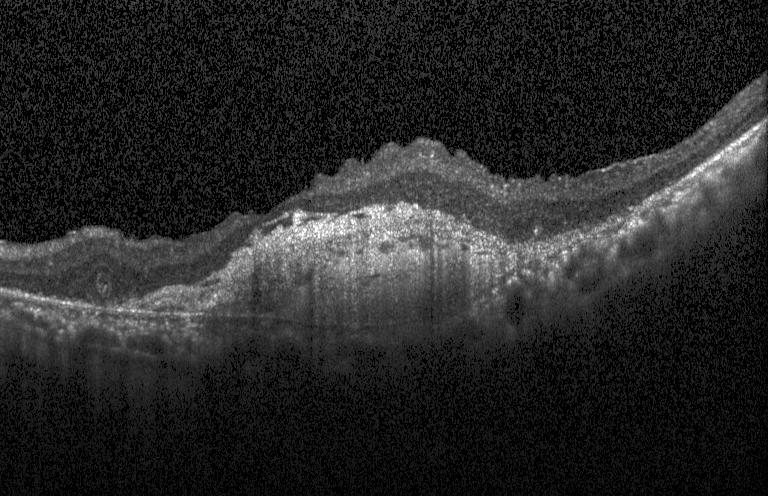
Assessment: choroidal neovascularization.